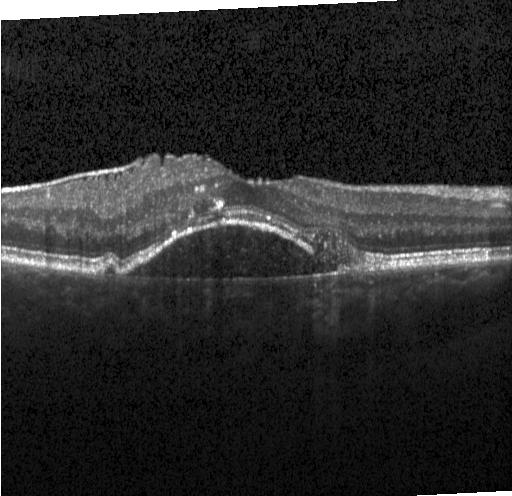
Spectral-domain optical coherence tomography · retinal OCT B-scan
Choroidal neovascularization (CNV).